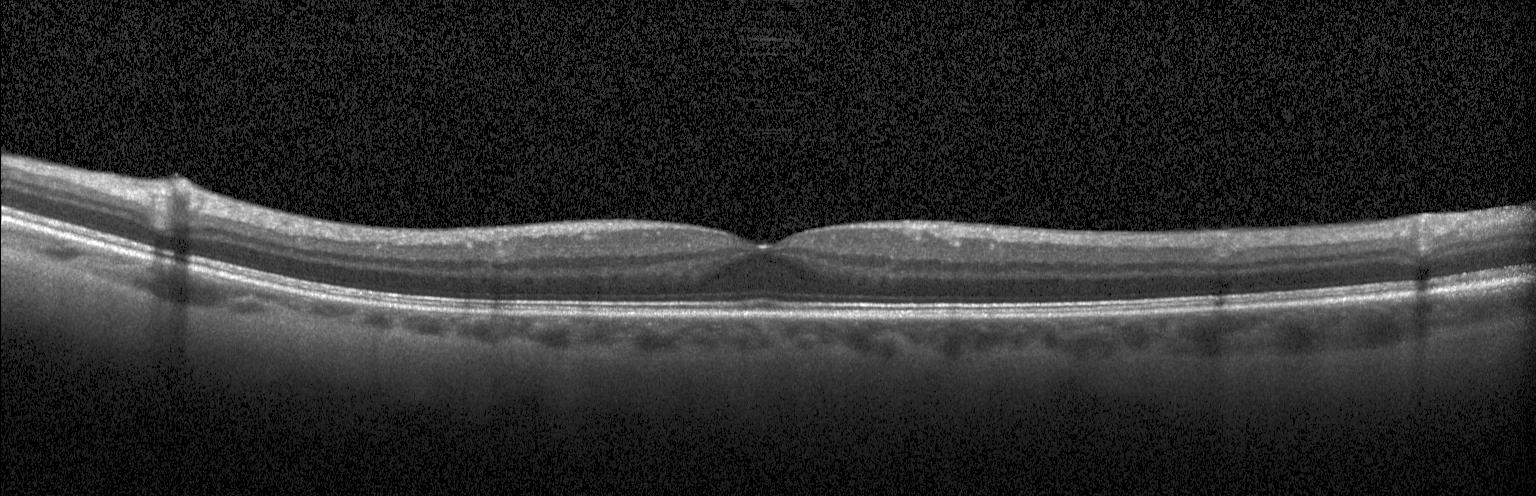
OCT line scan · through the macula — This B-scan demonstrates neither CNV, DME, nor drusen.